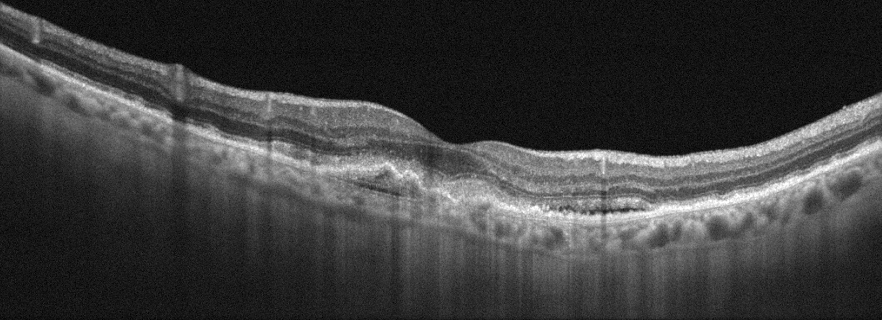 Instrument: Optovue Avanti RTVue XR, retinal OCT cross-section, fovea-centered.
This B-scan demonstrates AMD.